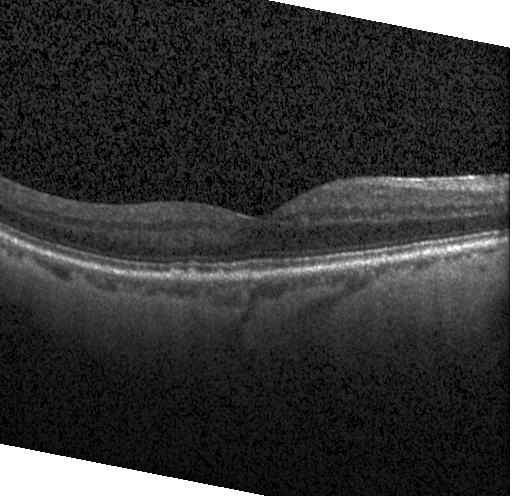
Drusen.